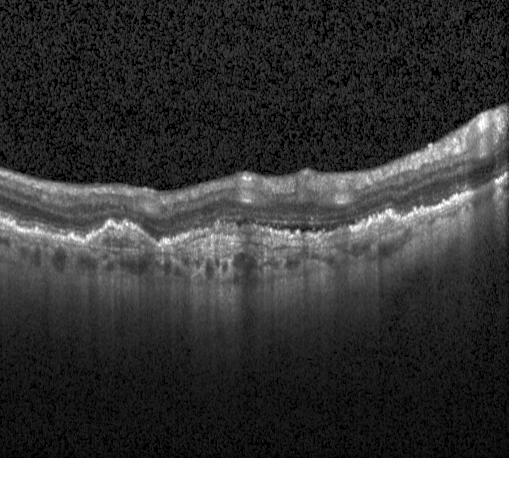

Spectral-domain OCT; horizontal scan through the fovea; retinal OCT cross-section — Finding: a choroidal neovascular membrane.